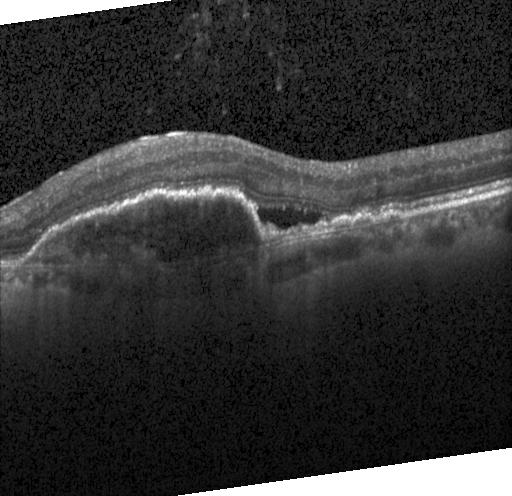 Spectral-domain optical coherence tomography. Retinal OCT cross-section
Dx: a choroidal neovascular membrane.